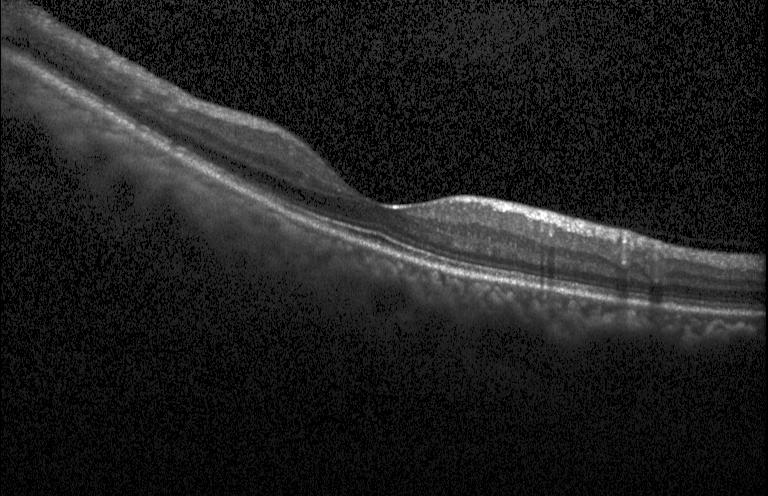
Retinal OCT B-scan; through the macula.
Impression: no choroidal neovascularization, no diabetic macular edema, and no drusen.